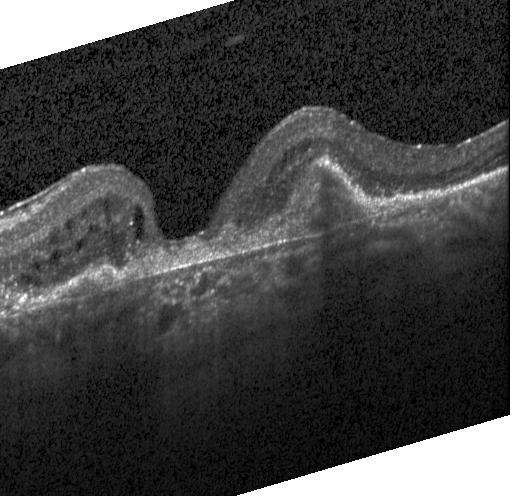 Spectral-domain OCT, OCT line scan — The scan shows a choroidal neovascular membrane.